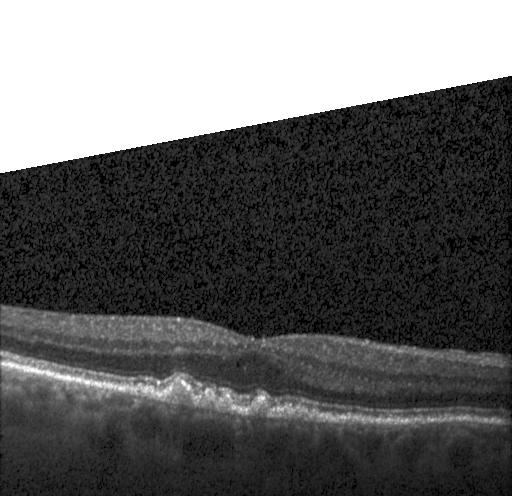
This B-scan demonstrates multiple drusen.